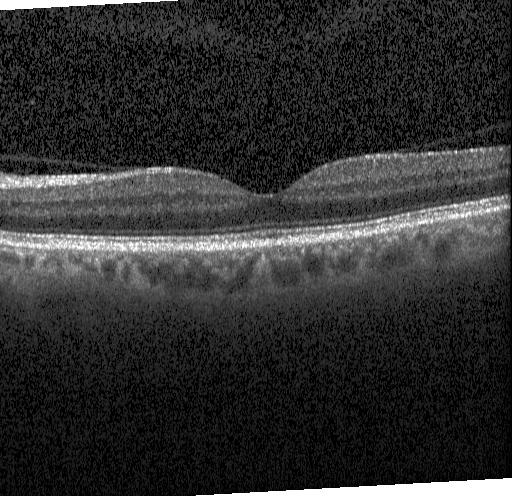

SD-OCT. Fovea-centered. OCT line scan — This B-scan demonstrates no evidence of choroidal neovascularization, diabetic macular edema, or drusen.